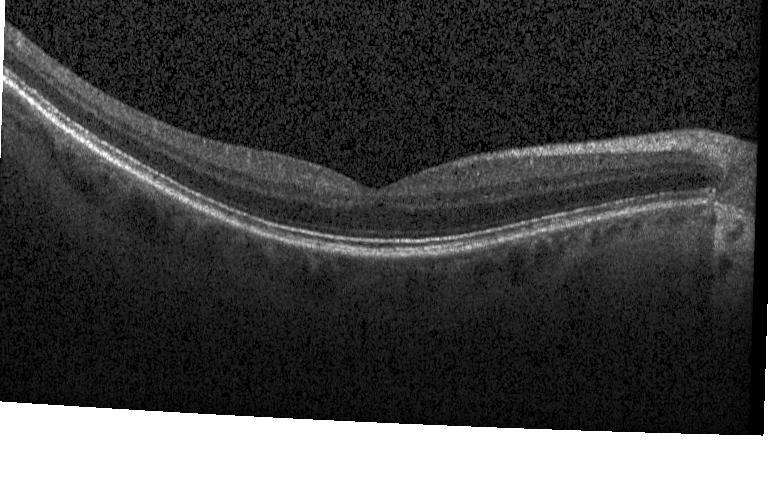
Acquired on a Heidelberg Spectralis; optical coherence tomography scan — This B-scan demonstrates no choroidal neovascularization, no diabetic macular edema, and no drusen.